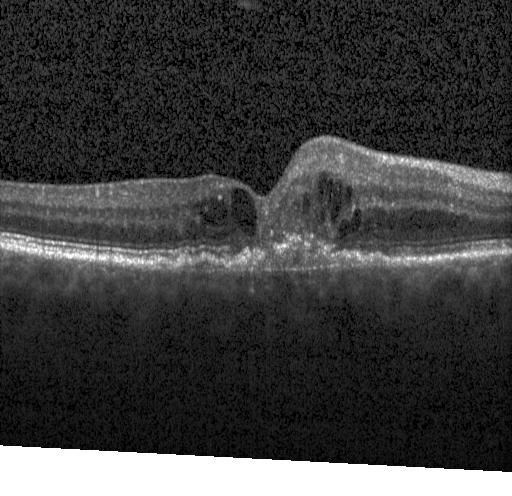

The scan shows a choroidal neovascular membrane.